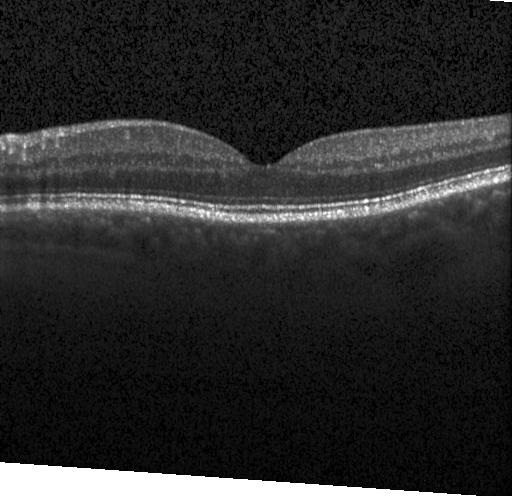
Heidelberg Spectralis; spectral-domain optical coherence tomography; OCT B-scan. Diagnosis: no CNV, no DME, and no drusen.